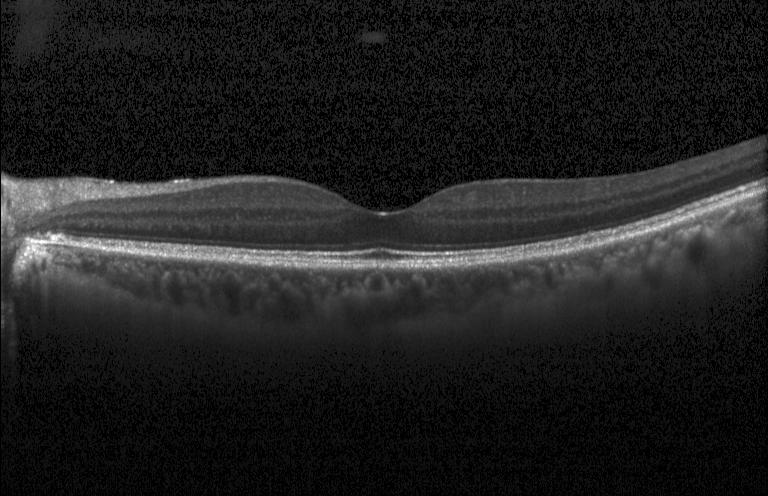

Instrument: Heidelberg Spectralis. Spectral-domain OCT. Retinal OCT B-scan. Macular scan. Assessment: no choroidal neovascularization, diabetic macular edema, or drusen.